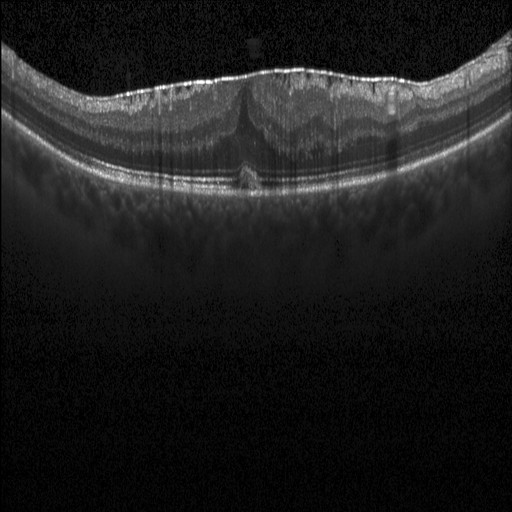
Optical coherence tomography scan, macular scan, spectral-domain OCT. The scan shows DME.